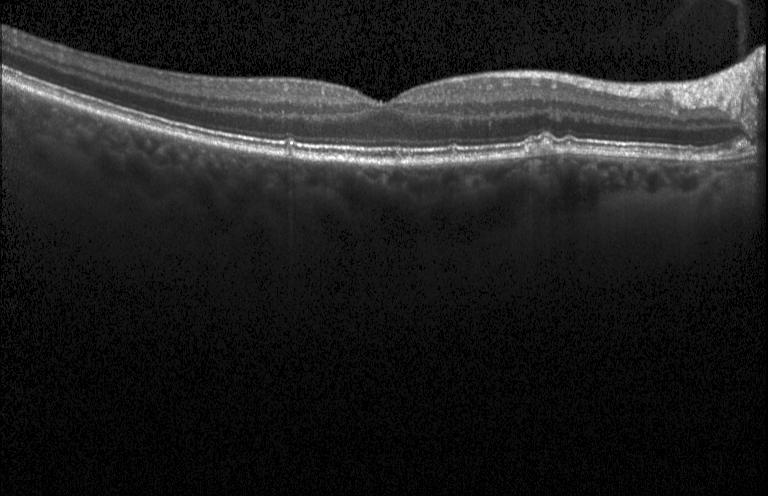 Horizontal scan through the fovea. Spectral-domain OCT. OCT B-scan. Acquired on a Heidelberg Spectralis. Drusen.